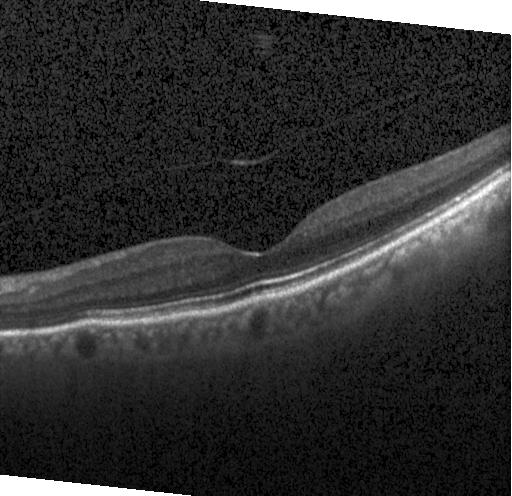

Centered on the fovea · acquired on a Heidelberg Spectralis · retinal OCT B-scan — This B-scan demonstrates no choroidal neovascularization, diabetic macular edema, or drusen.